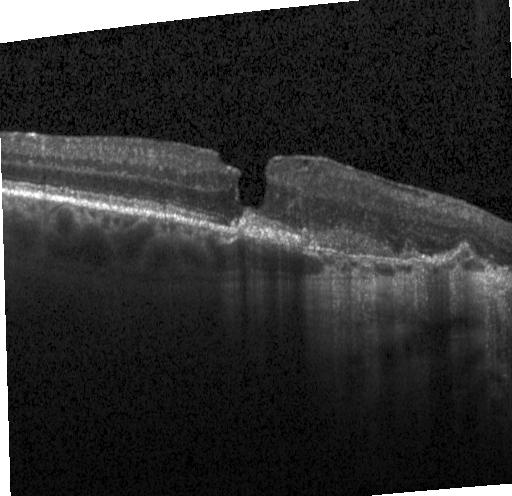
OCT B-scan showing a choroidal neovascular membrane.